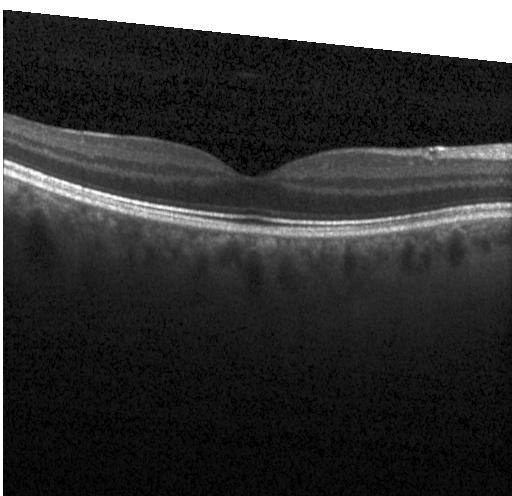 Centered on the fovea; Heidelberg Spectralis OCT system; retinal OCT cross-section.
Dx: no CNV, DME, or drusen.